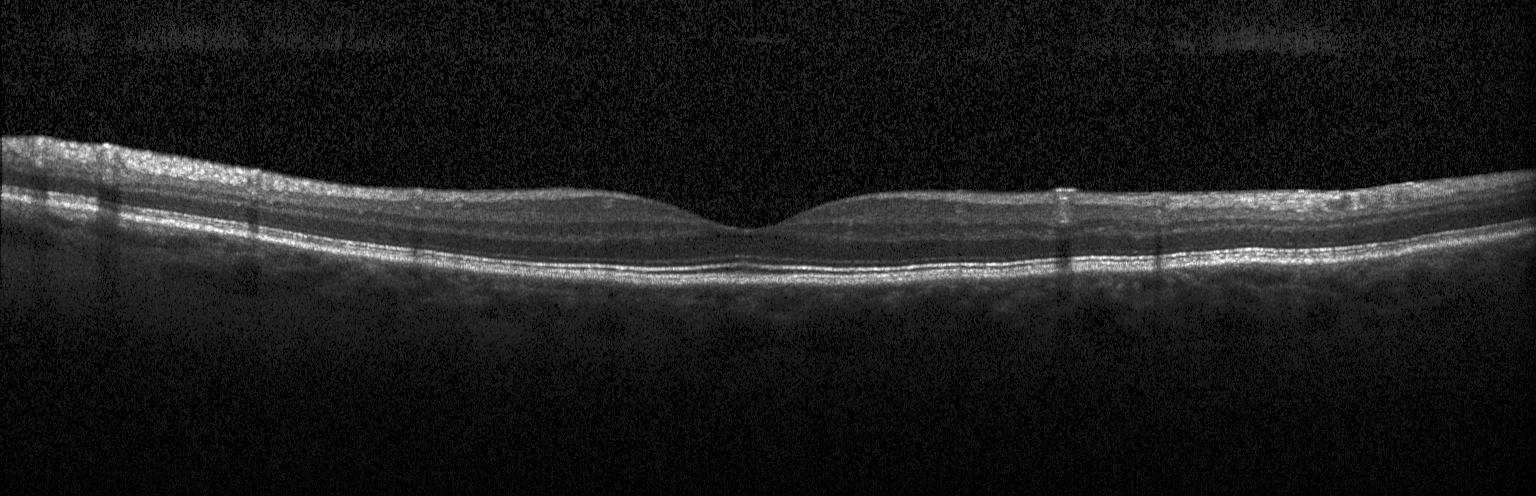

Finding: neither choroidal neovascularization, diabetic macular edema, nor drusen.